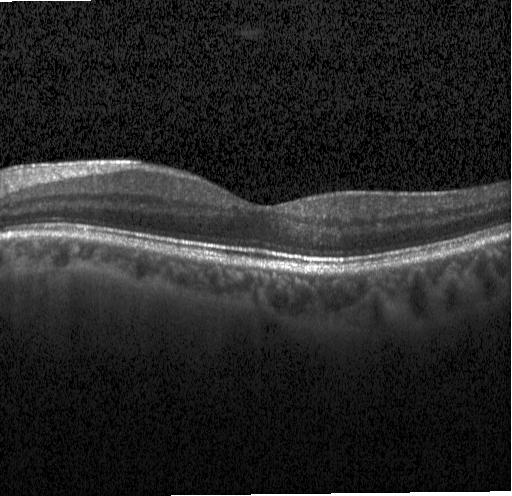
Assessment: neither choroidal neovascularization, diabetic macular edema, nor drusen.